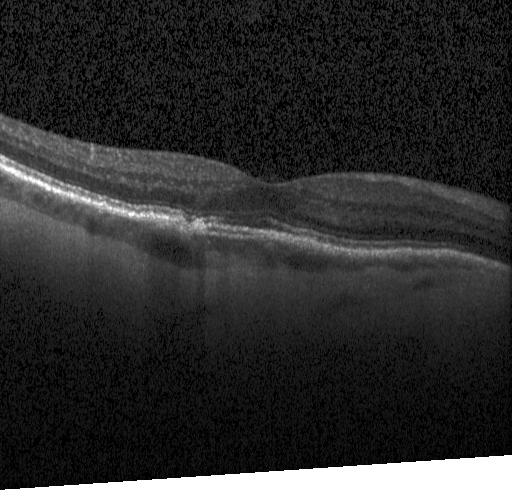 Macular scan · OCT B-scan · acquired on a Heidelberg Spectralis · SD-OCT
Assessment: multiple drusen.